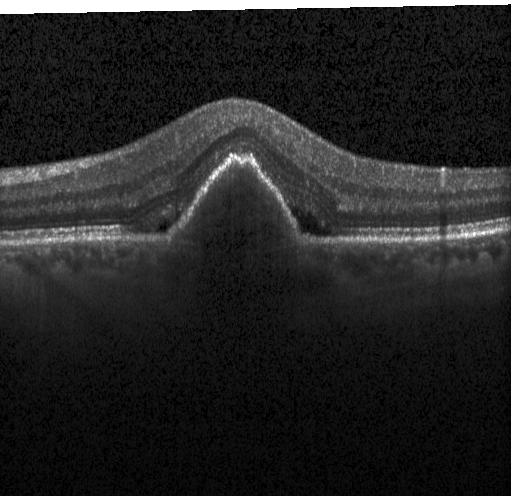
Centered on the fovea, retinal OCT B-scan, spectral-domain OCT, Heidelberg Spectralis — Choroidal neovascularization.